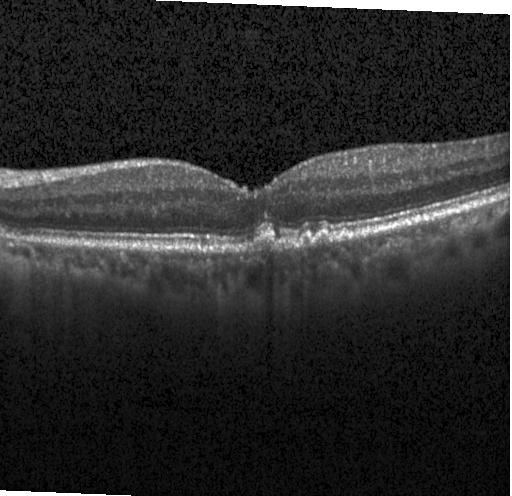
Macular OCT demonstrating drusen.